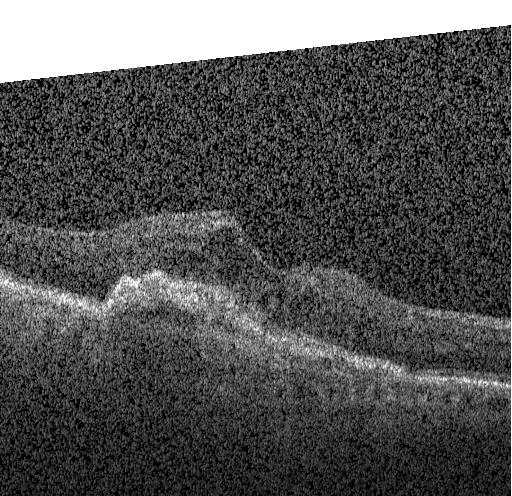

OCT B-scan. Assessment: a choroidal neovascular membrane.